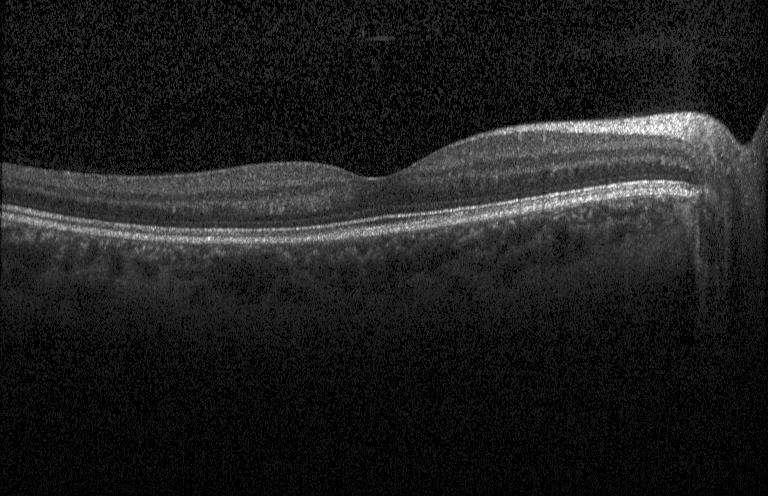

OCT line scan; instrument: Heidelberg Spectralis; spectral-domain OCT.
The scan shows no choroidal neovascularization, no diabetic macular edema, and no drusen.